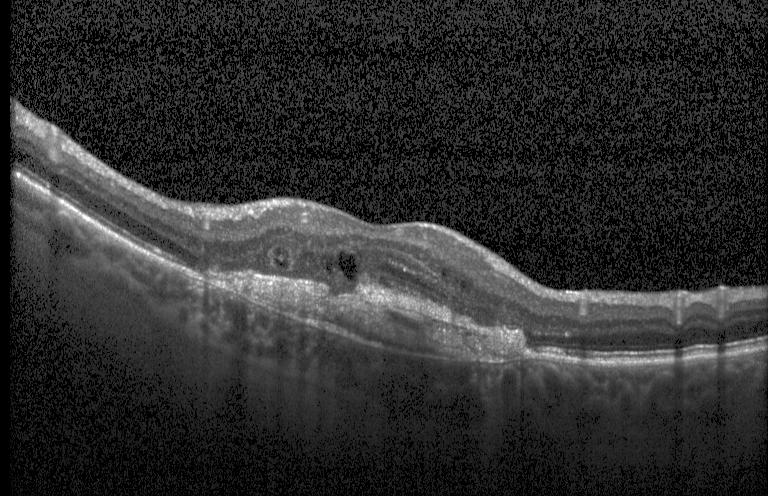 Heidelberg Spectralis, retinal OCT B-scan — The scan shows a choroidal neovascular membrane.